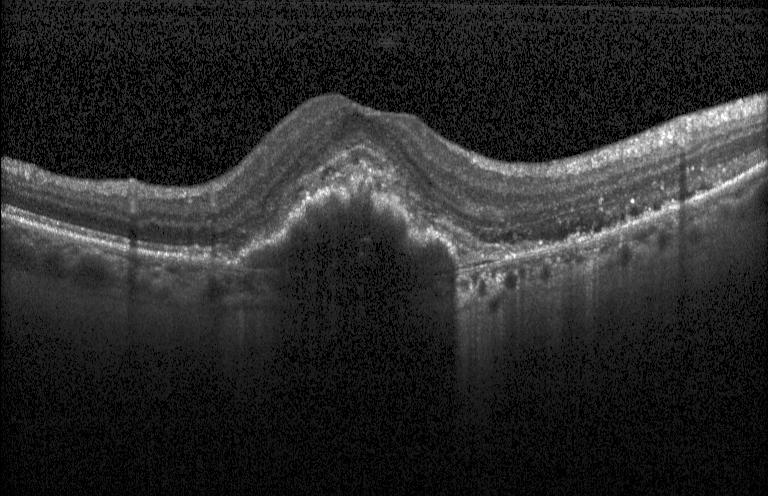
Finding: a choroidal neovascular membrane.